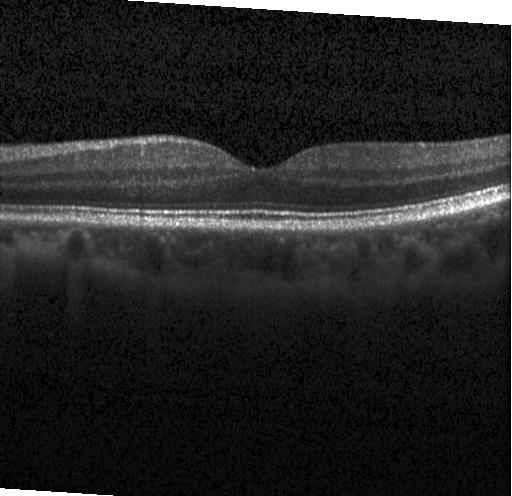

Dx: neither choroidal neovascularization, diabetic macular edema, nor drusen.